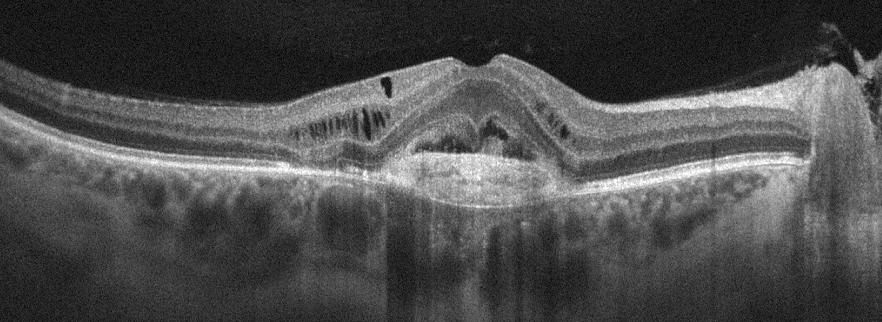
Retinal OCT B-scan — Diagnosis: AMD.